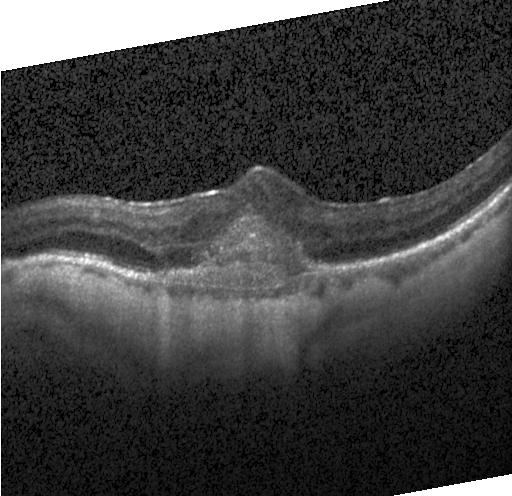

Spectral-domain optical coherence tomography. OCT B-scan. Through the macula — Assessment: a choroidal neovascular membrane.